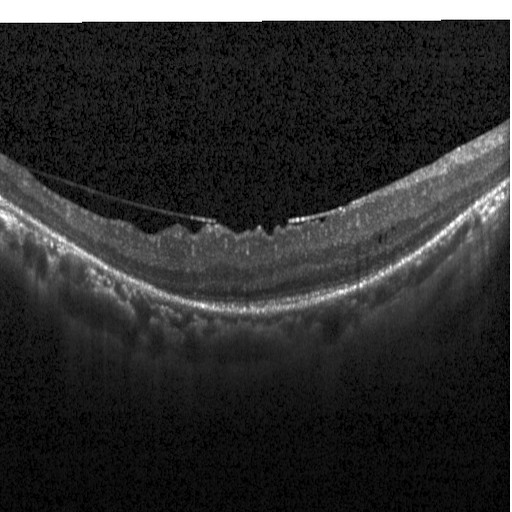 Optical coherence tomography scan; acquired on a Heidelberg Spectralis
Diagnosis: DME.